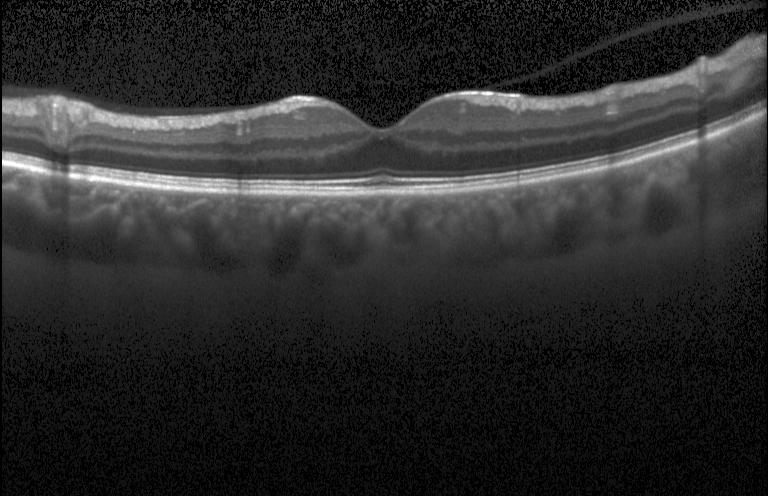
Spectral-domain optical coherence tomography; horizontal scan through the fovea; OCT line scan; Heidelberg Spectralis. Macular OCT: no CNV, DME, or drusen.